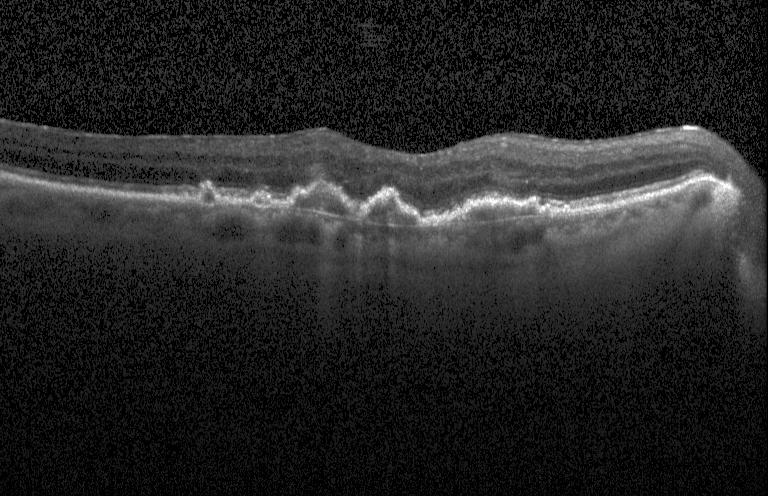
Heidelberg Spectralis OCT system, optical coherence tomography scan
OCT finding: CNV.